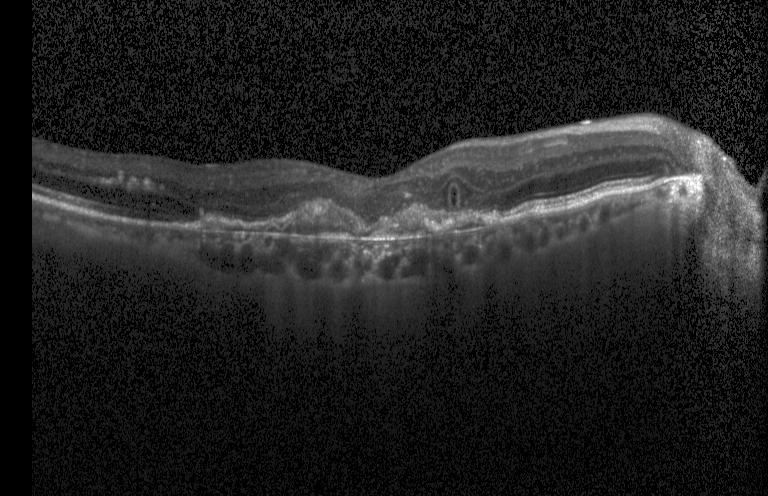
Diagnosis: a choroidal neovascular membrane.